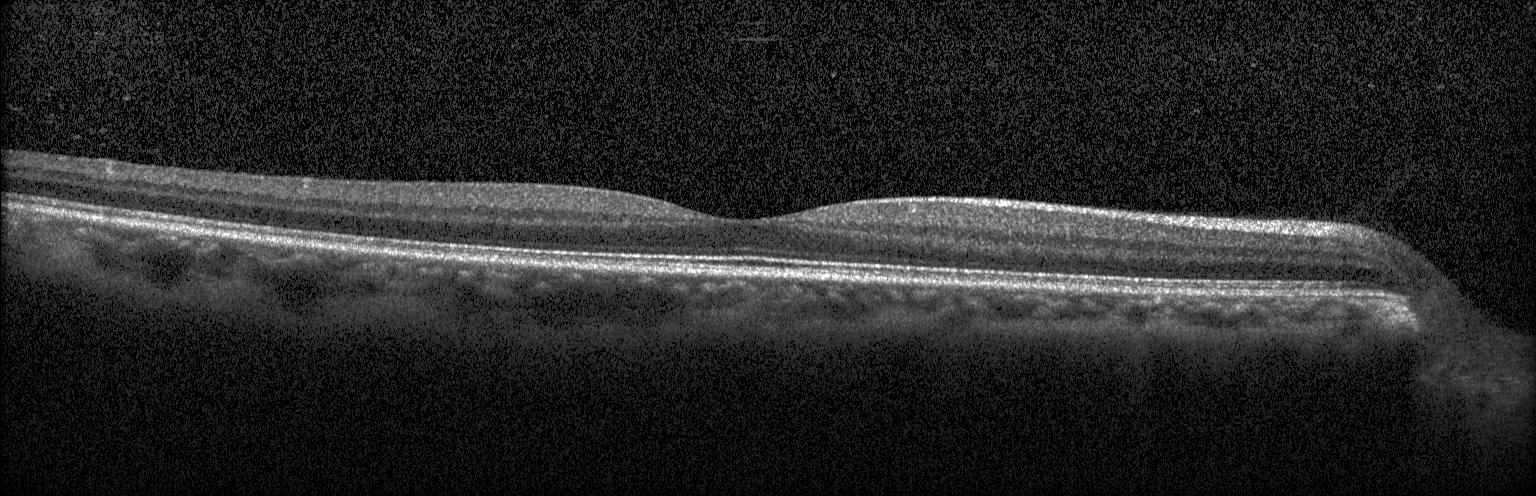

Optical coherence tomography B-scan, instrument: Heidelberg Spectralis
Finding: no choroidal neovascularization, no diabetic macular edema, and no drusen.